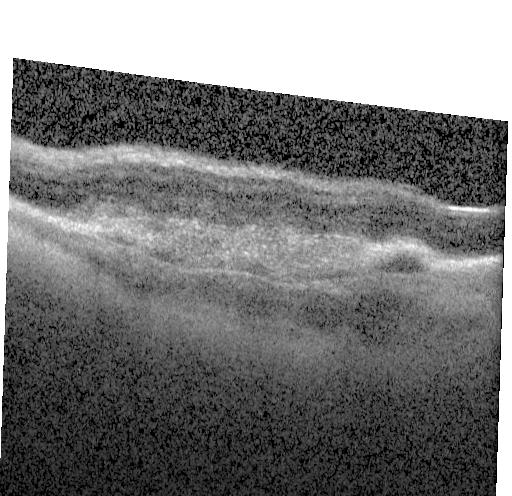
Centered on the fovea. Optical coherence tomography scan. Spectral-domain OCT. Impression: CNV.